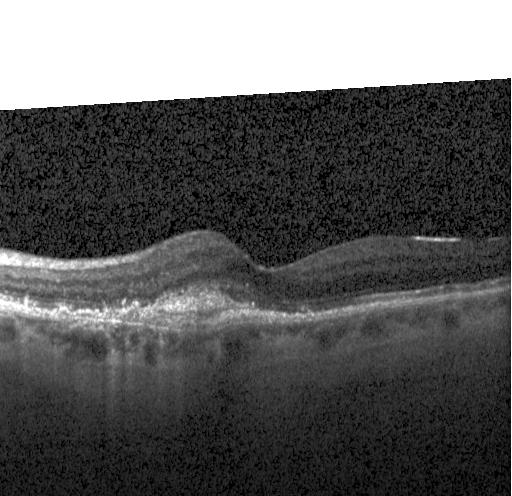

Diagnosis: a choroidal neovascular membrane.